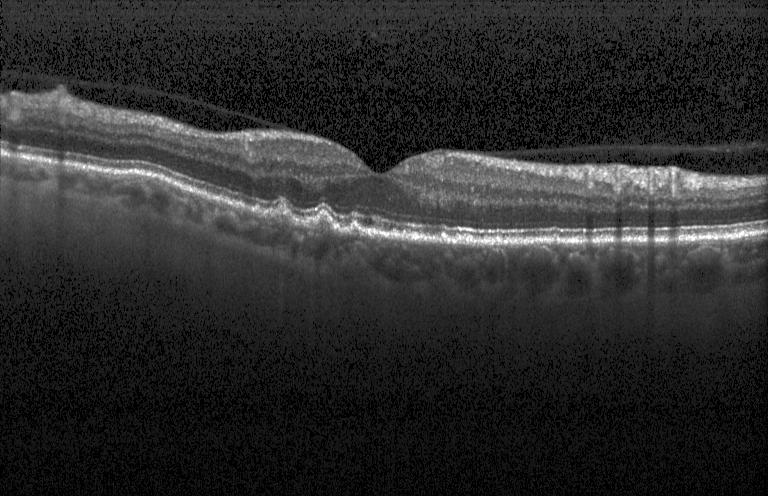

Dx: drusen.